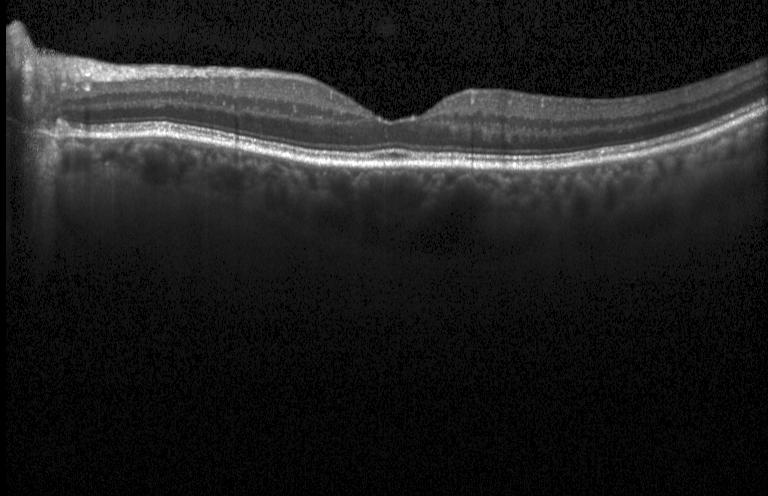

OCT B-scan.
Diagnosis: no CNV, DME, or drusen.